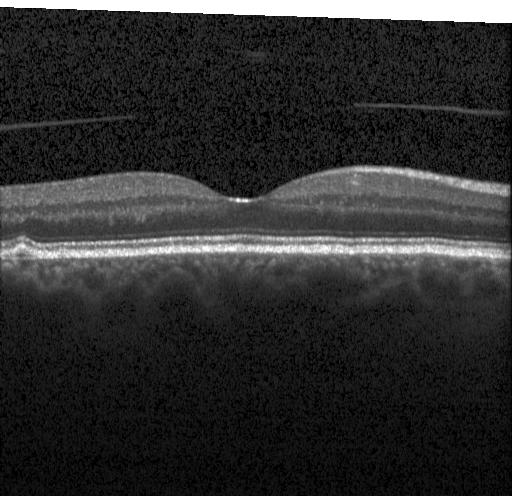

Retinal OCT B-scan · Heidelberg Spectralis OCT system.
Sub-RPE drusenoid deposits.